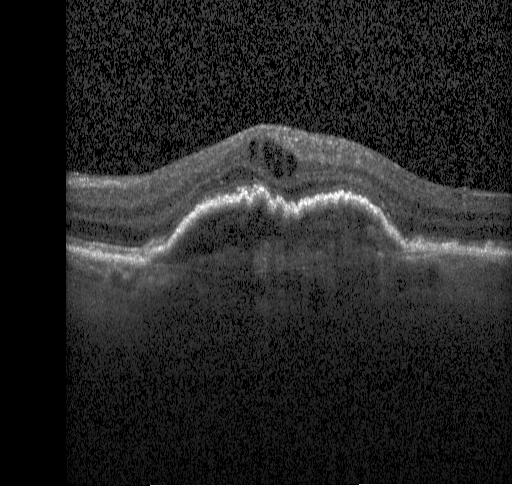
OCT B-scan, instrument: Heidelberg Spectralis
Diagnosis: CNV.